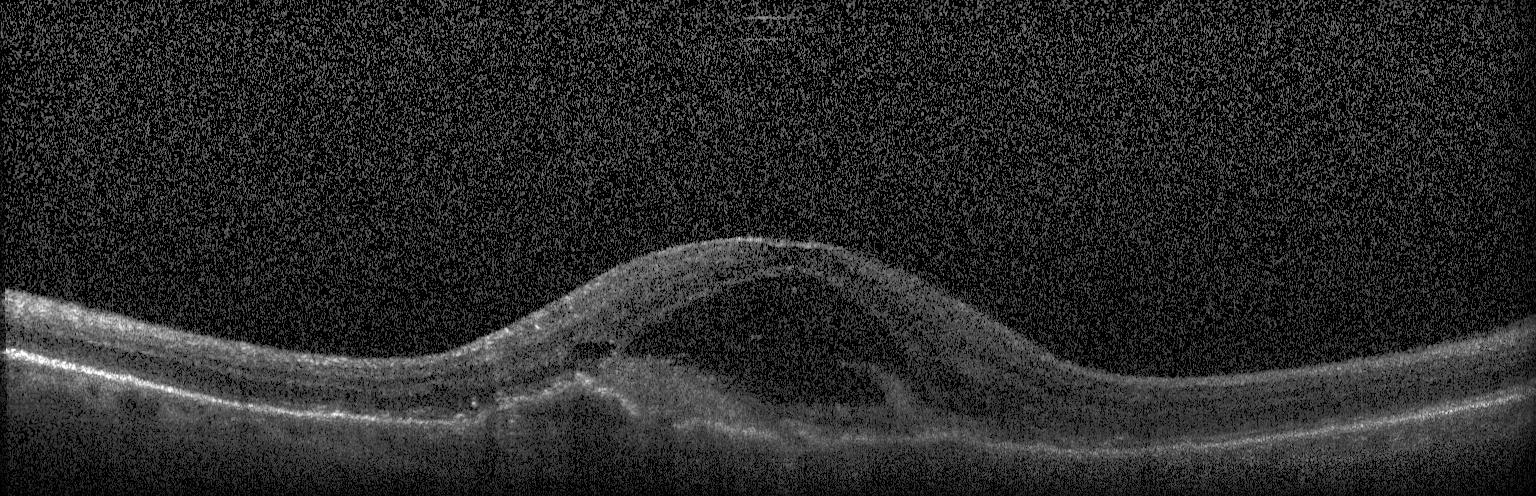

Centered on the fovea · retinal OCT cross-section · spectral-domain OCT · acquired on a Heidelberg Spectralis.
Diagnosis: choroidal neovascularization (CNV).